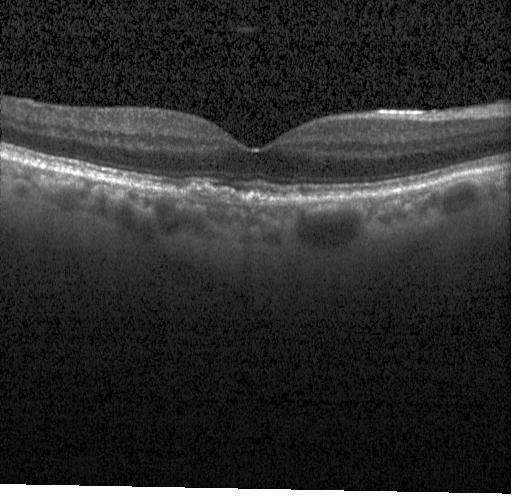 Retinal OCT B-scan
The scan shows sub-RPE drusenoid deposits.